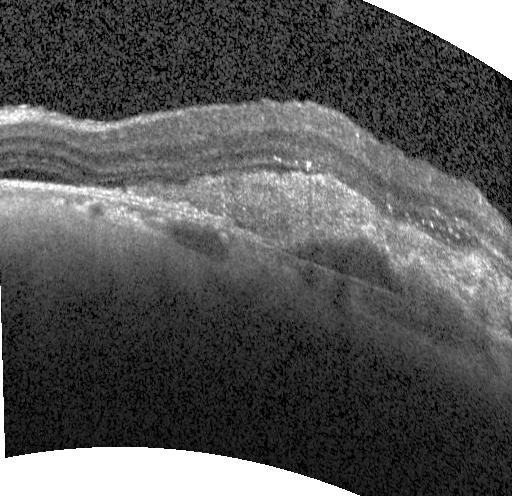

Macular OCT: a choroidal neovascular membrane.